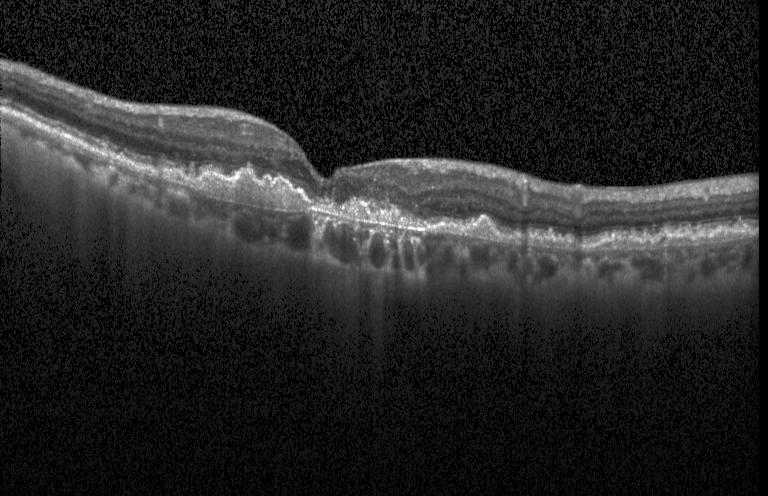

Optical coherence tomography scan · fovea-centered — Impression: a choroidal neovascular membrane.